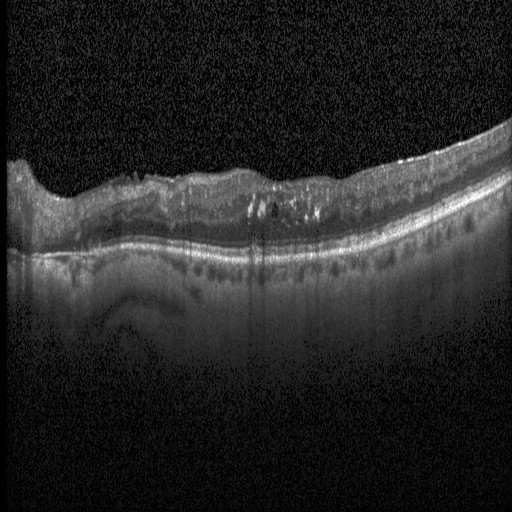 OCT finding: DME.